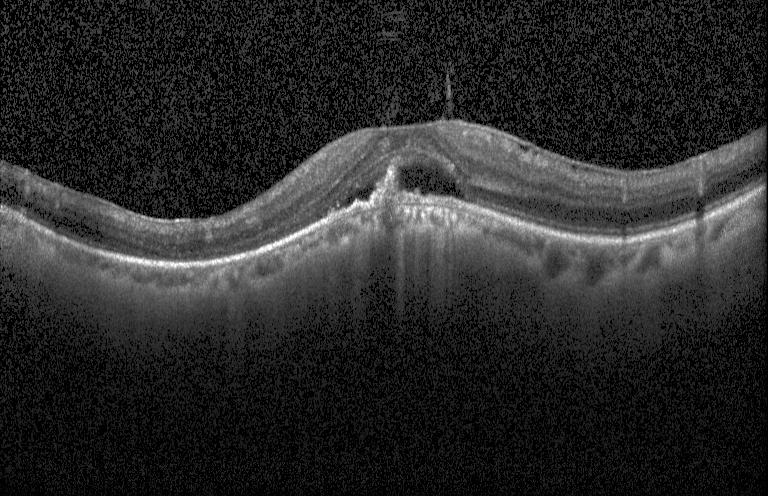
Heidelberg Spectralis OCT system · centered on the fovea · spectral-domain OCT · optical coherence tomography scan — Macular OCT: a choroidal neovascular membrane.